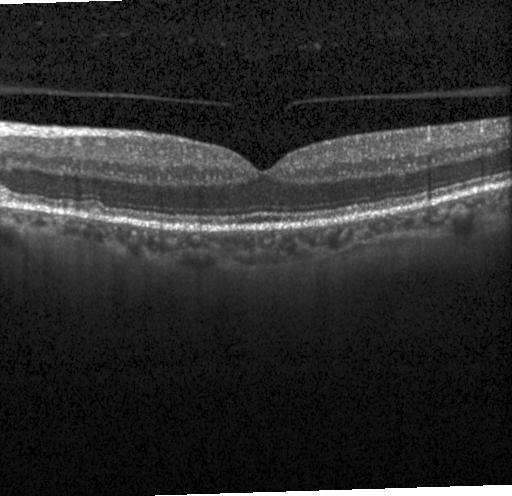

Acquired on a Heidelberg Spectralis. Horizontal scan through the fovea. Retinal OCT B-scan. The scan shows multiple drusen.